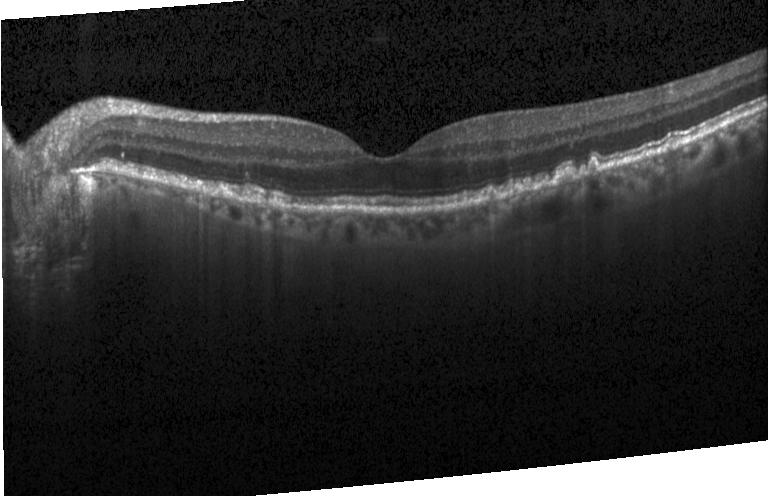

The scan shows drusen.